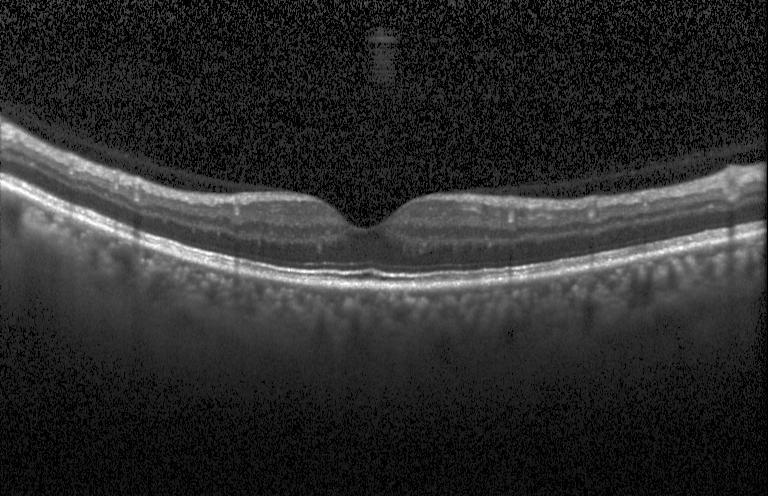
OCT B-scan.
This B-scan demonstrates no evidence of CNV, DME, or drusen.